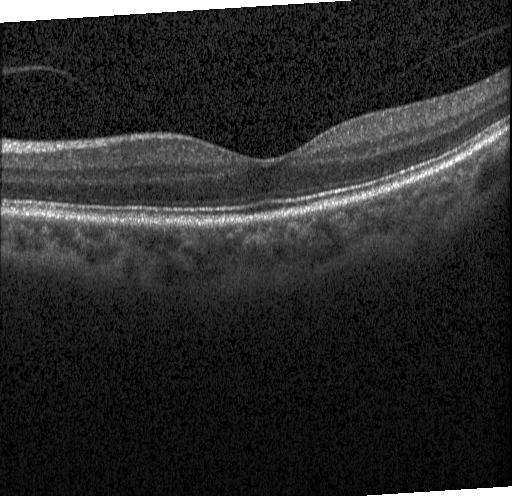

Retinal OCT cross-section showing no choroidal neovascularization, diabetic macular edema, or drusen.